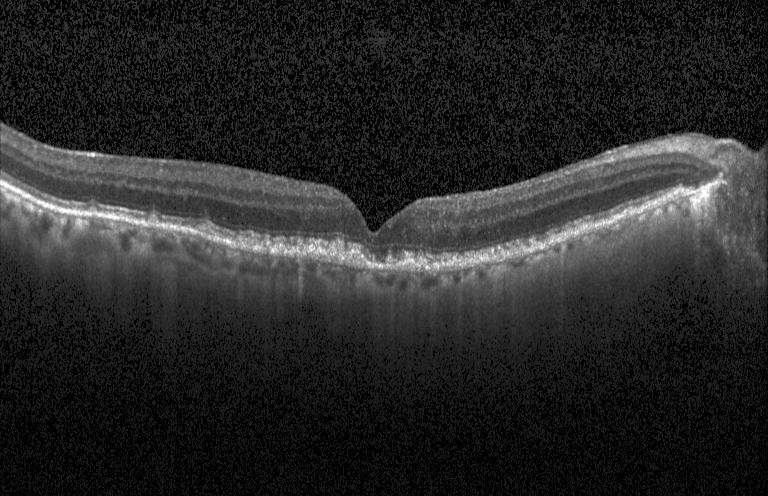

Impression: drusen.